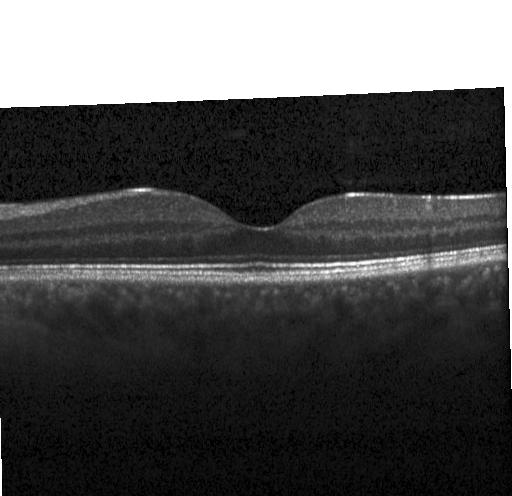
Instrument: Heidelberg Spectralis · fovea-centered · retinal OCT B-scan — Impression: no CNV, no DME, and no drusen.